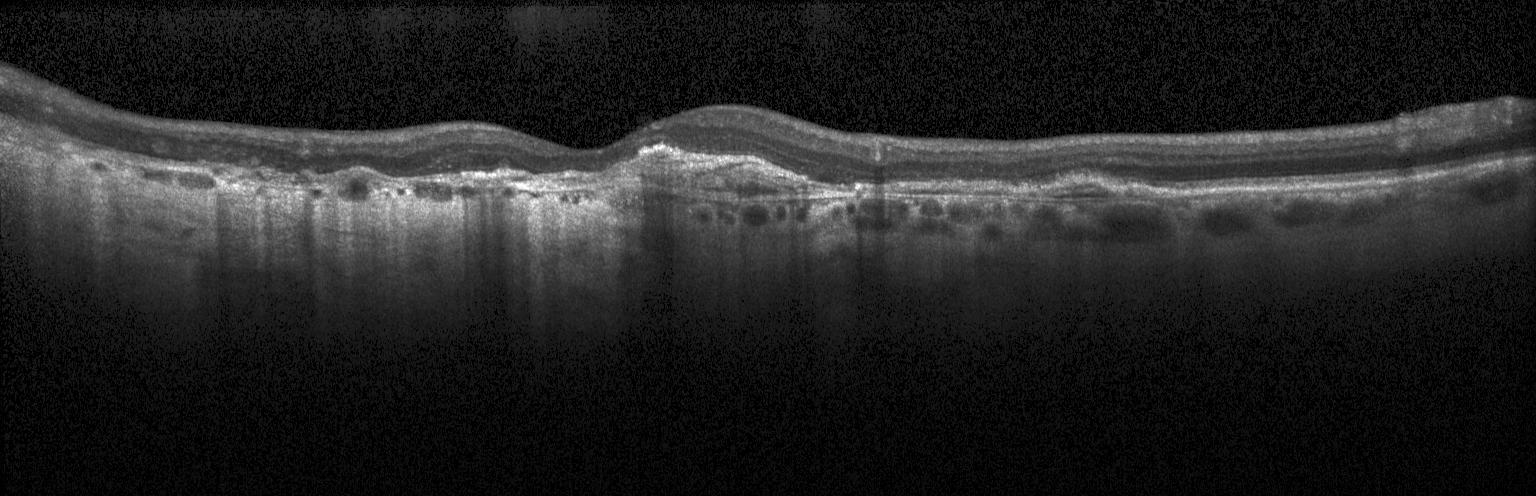
Retinal OCT B-scan.
Diagnosis: a choroidal neovascular membrane.